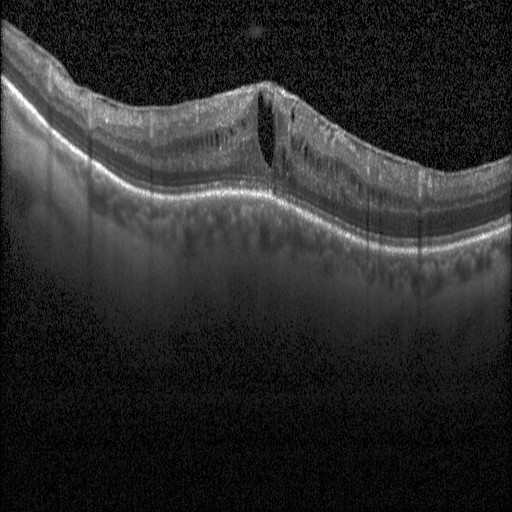
OCT line scan. Through the macula. Acquired on a Heidelberg Spectralis
Dx: DME.